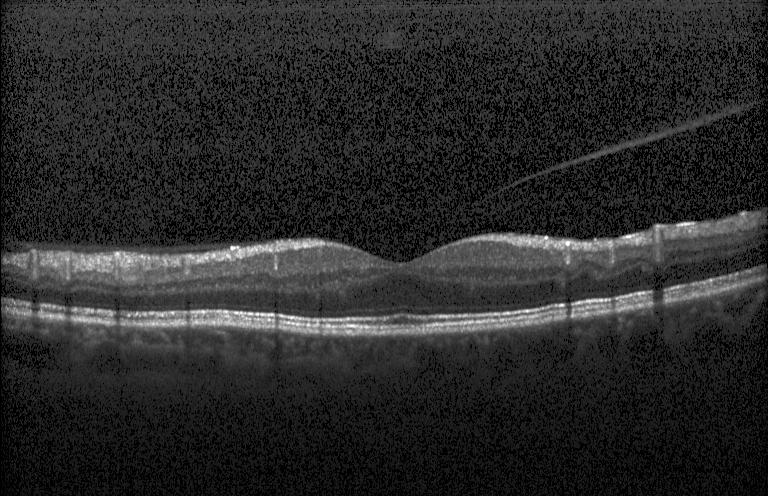

Neither choroidal neovascularization, diabetic macular edema, nor drusen.